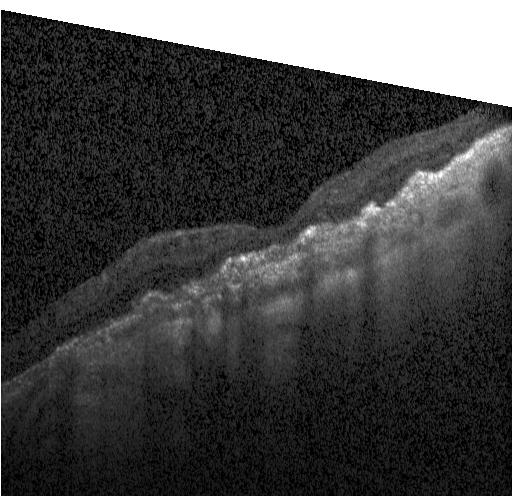 Diagnosis: CNV.